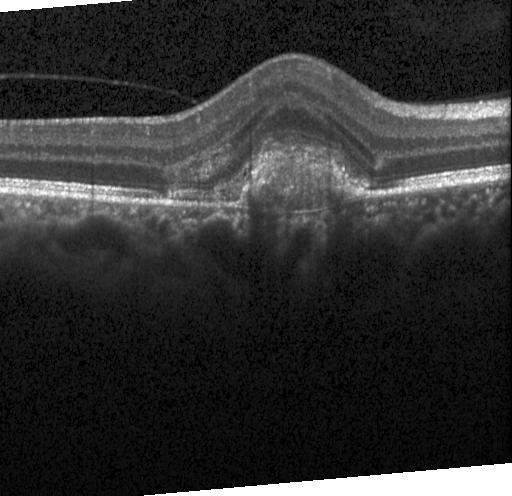 Through the macula · retinal OCT B-scan
Impression: choroidal neovascularization (CNV).